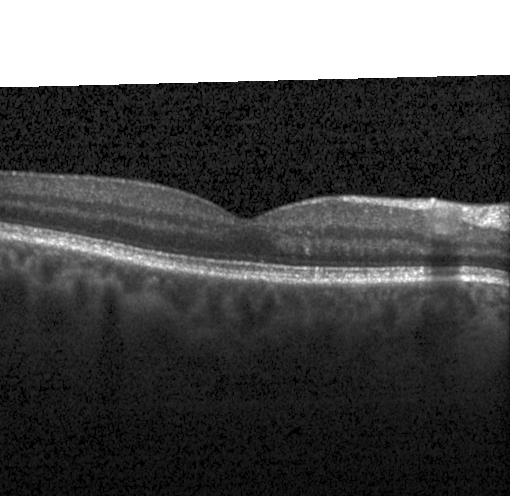

Retinal OCT cross-section showing no choroidal neovascularization, no diabetic macular edema, and no drusen.